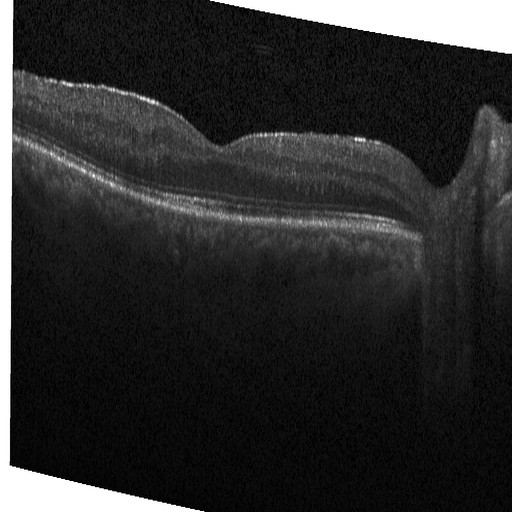

Retinal OCT cross-section, macular scan, spectral-domain OCT.
Diagnosis: diabetic macular edema (DME).